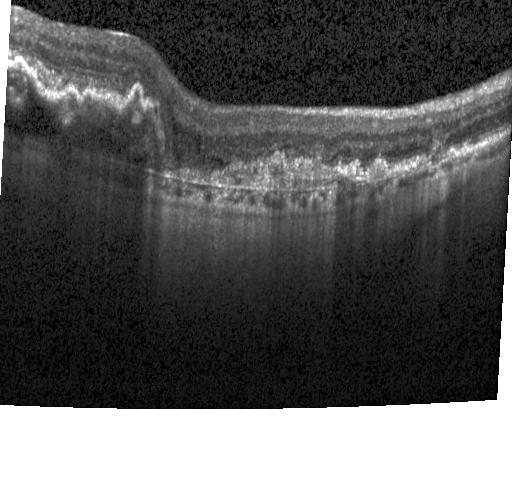 Heidelberg Spectralis · optical coherence tomography B-scan
The scan shows choroidal neovascularization (CNV).